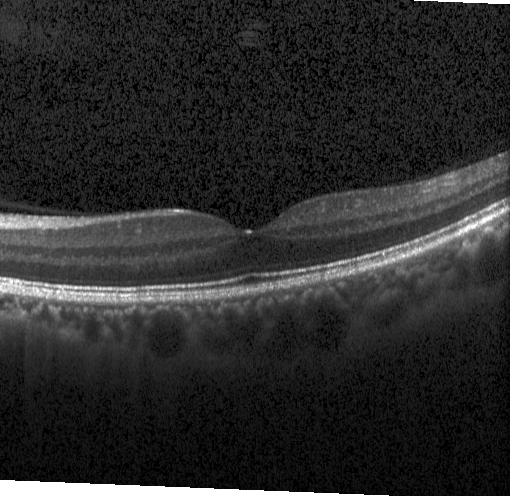 OCT B-scan showing no choroidal neovascularization, no diabetic macular edema, and no drusen.